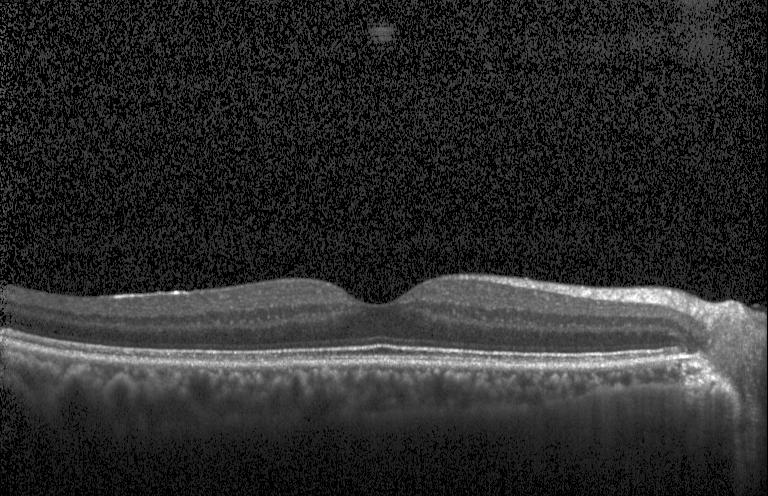

Acquired on a Heidelberg Spectralis. Retinal OCT B-scan.
Finding: no CNV, DME, or drusen.